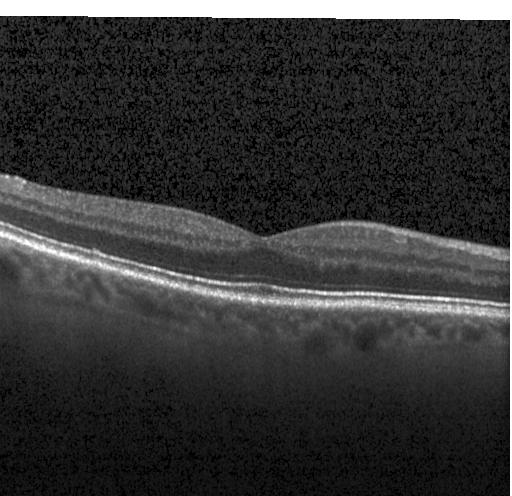

Optical coherence tomography B-scan, through the macula, spectral-domain optical coherence tomography — OCT finding: neither CNV, DME, nor drusen.